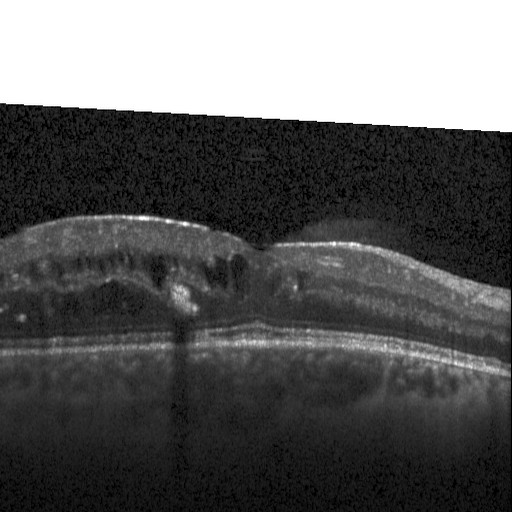 Macular scan; spectral-domain OCT; optical coherence tomography scan; acquired on a Heidelberg Spectralis.
Macular OCT: diabetic macular edema (DME).